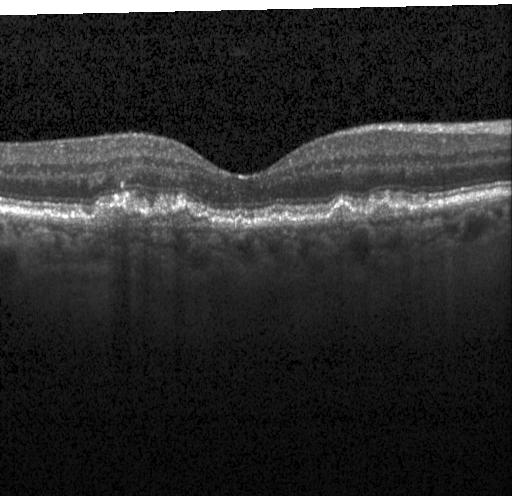 Finding: a choroidal neovascular membrane.